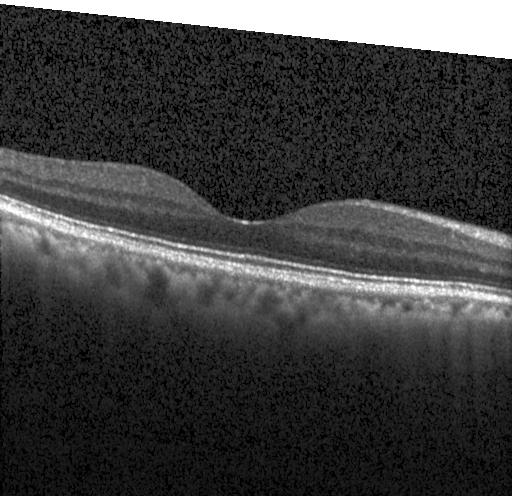 Assessment: no choroidal neovascularization, no diabetic macular edema, and no drusen.